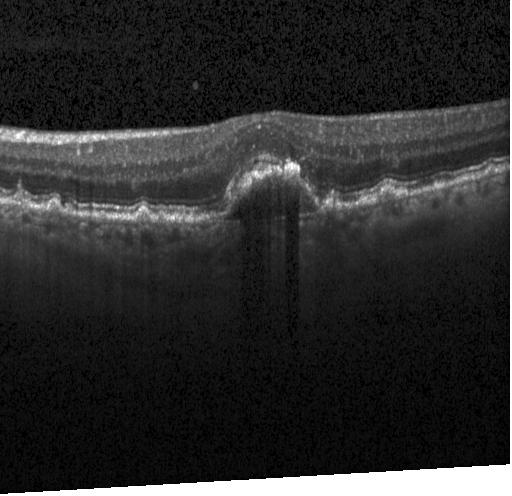 Optical coherence tomography B-scan.
Impression: choroidal neovascularization (CNV).